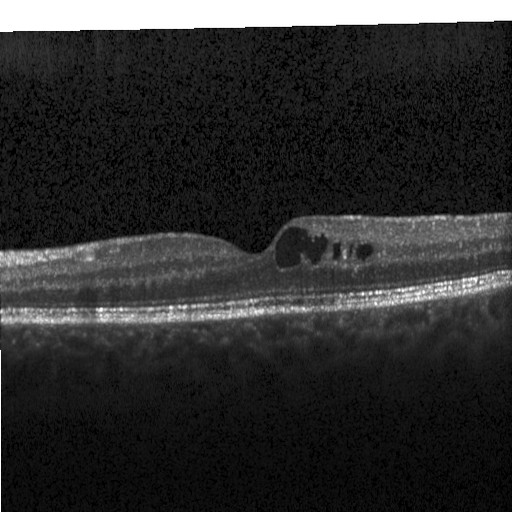
Optical coherence tomography B-scan. Spectral-domain optical coherence tomography. Heidelberg Spectralis.
Impression: DME.